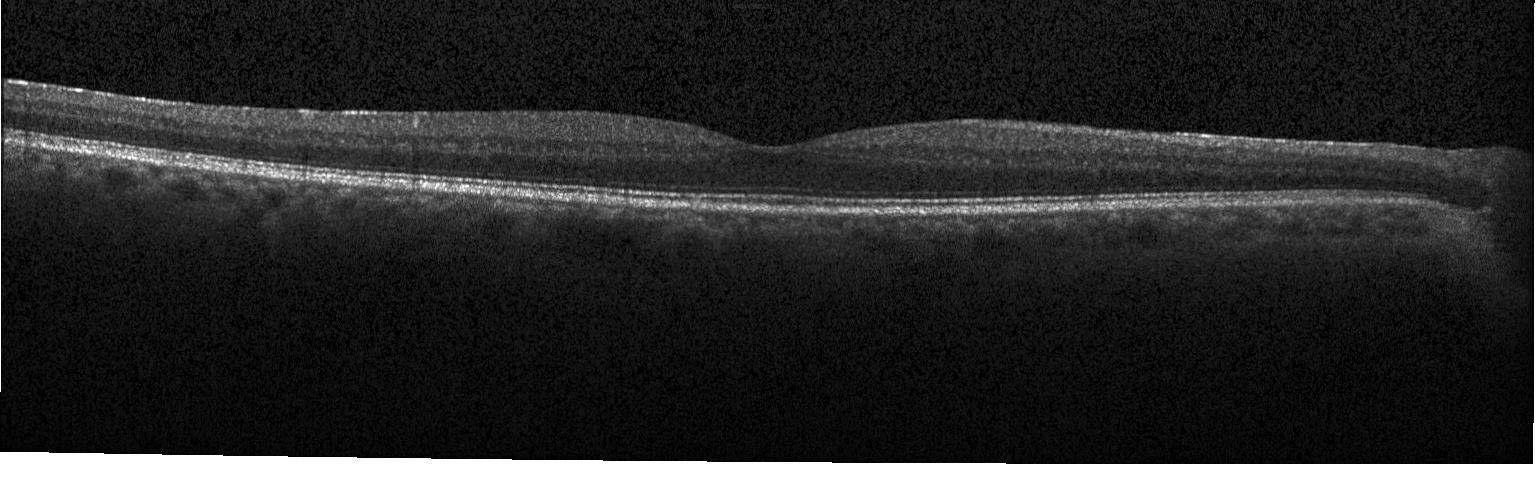
Instrument: Heidelberg Spectralis · optical coherence tomography B-scan · fovea-centered · SD-OCT
No CNV, DME, or drusen.